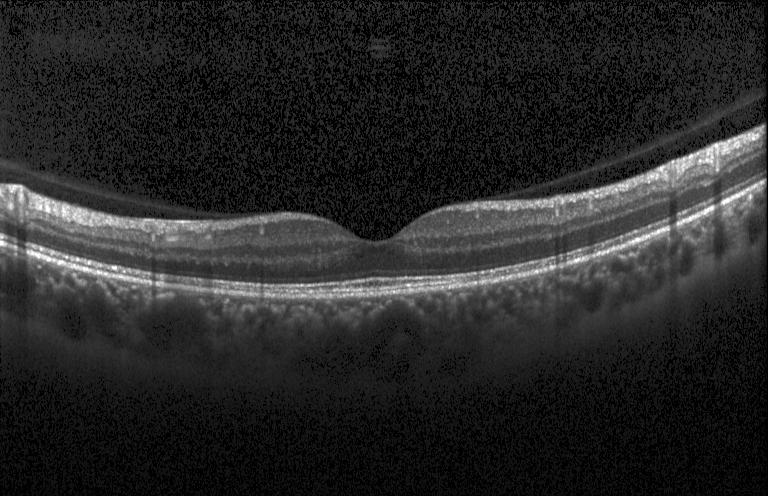

This B-scan demonstrates neither choroidal neovascularization, diabetic macular edema, nor drusen.